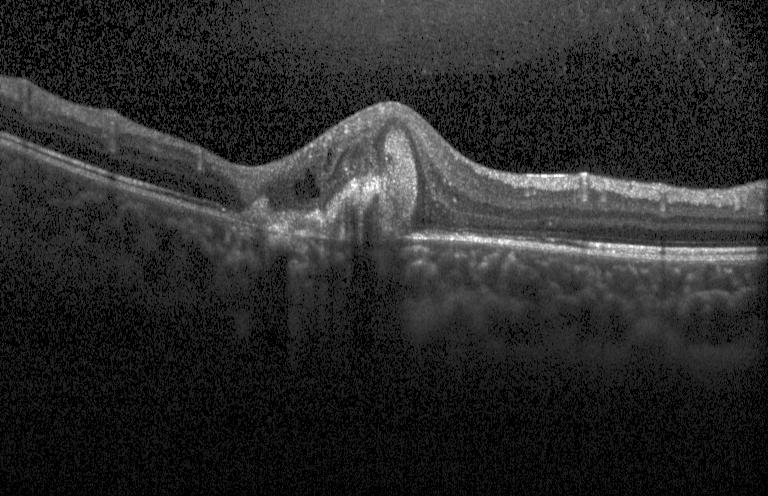 Optical coherence tomography scan · spectral-domain OCT · instrument: Heidelberg Spectralis.
Choroidal neovascularization.